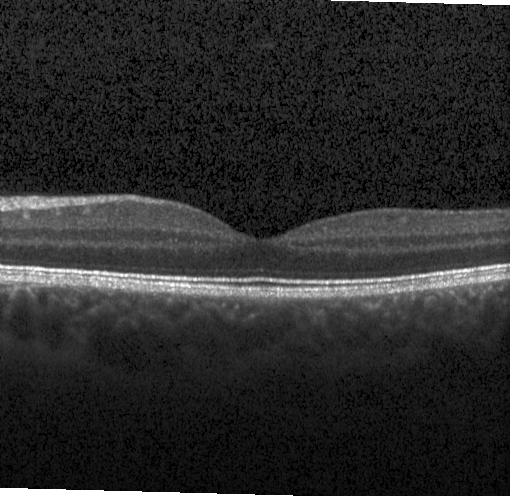

Retinal OCT B-scan
The scan shows no choroidal neovascularization, no diabetic macular edema, and no drusen.